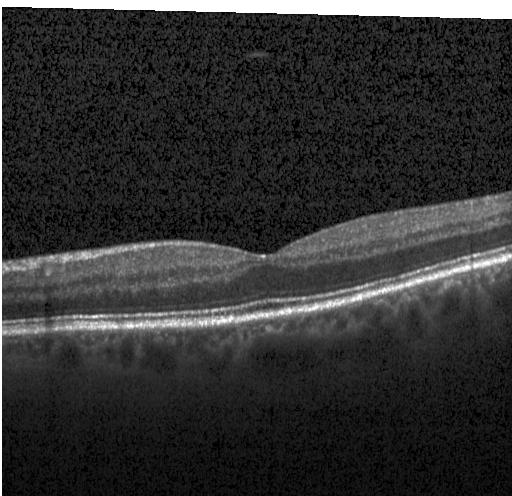

Impression: no choroidal neovascularization, no diabetic macular edema, and no drusen.